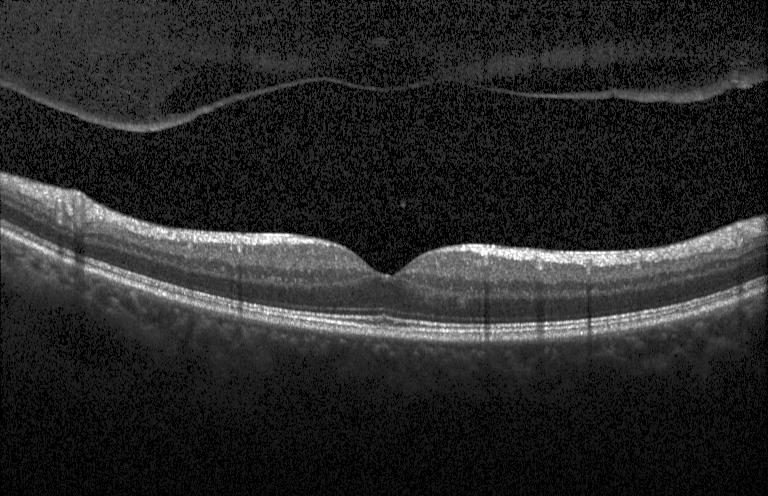 Macular OCT: no evidence of choroidal neovascularization, diabetic macular edema, or drusen.